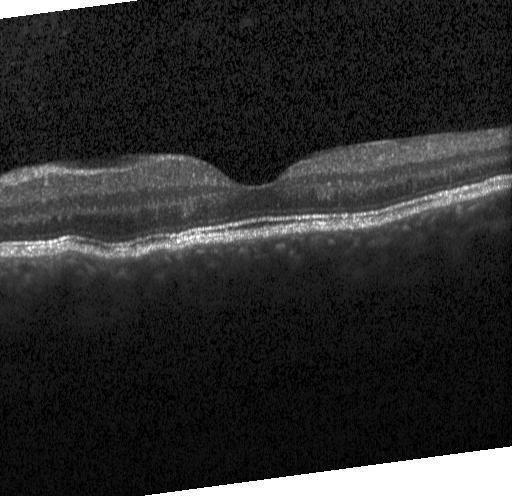 Retinal OCT B-scan · spectral-domain optical coherence tomography · macular scan · instrument: Heidelberg Spectralis. OCT finding: no choroidal neovascularization, no diabetic macular edema, and no drusen.